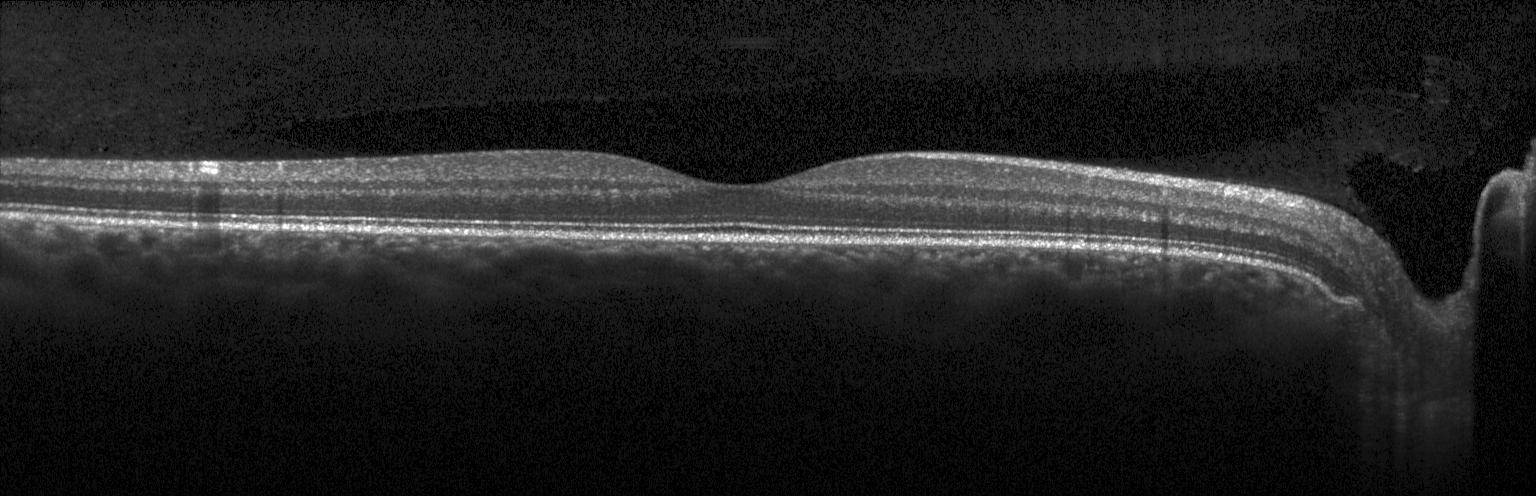 Dx: no choroidal neovascularization, diabetic macular edema, or drusen.